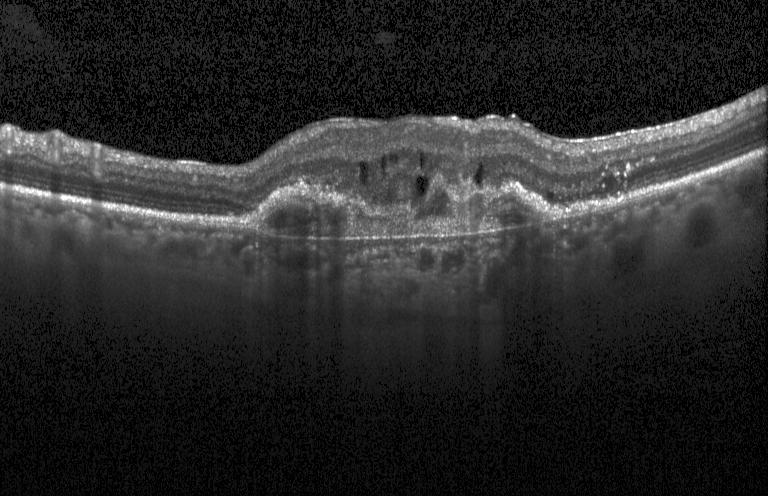
Spectral-domain optical coherence tomography, retinal OCT B-scan, horizontal scan through the fovea, Heidelberg Spectralis.
Diagnosis: a choroidal neovascular membrane.